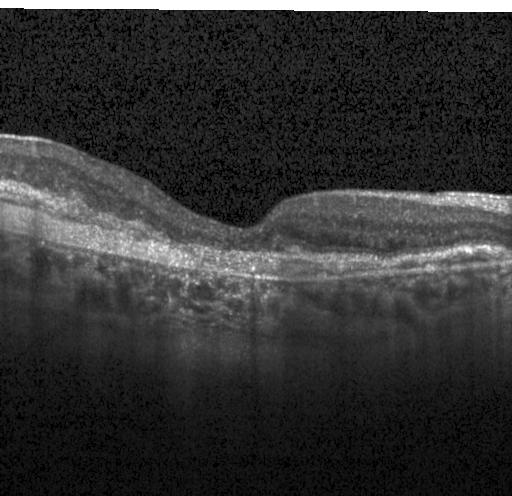 Retinal OCT cross-section.
Impression: a choroidal neovascular membrane.